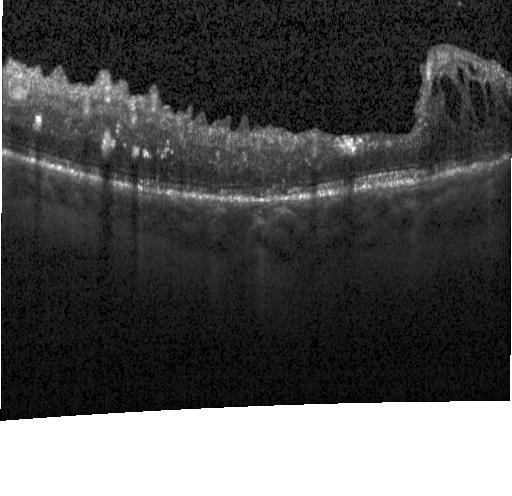 Spectral-domain OCT B-scan: DME.